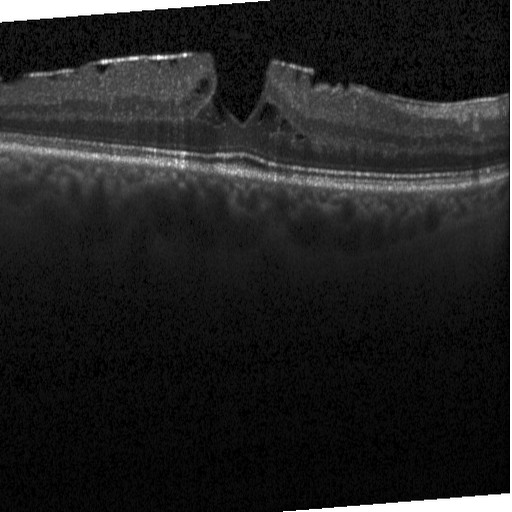
OCT line scan.
Finding: DME.